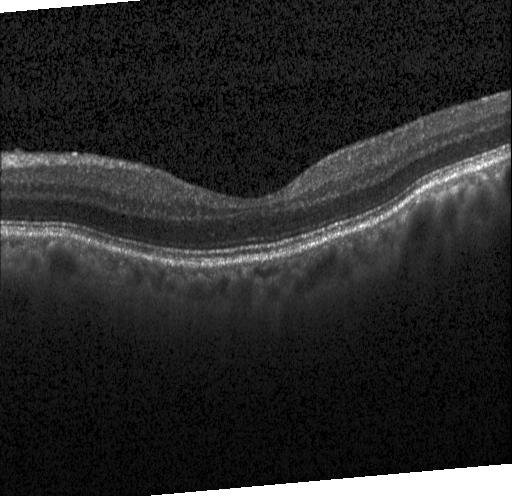
Retinal OCT B-scan; centered on the fovea; spectral-domain OCT
Diagnosis: no CNV, DME, or drusen.